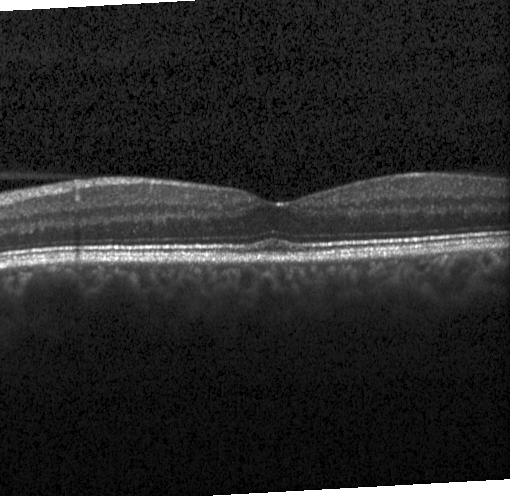
Finding: no evidence of choroidal neovascularization, diabetic macular edema, or drusen.